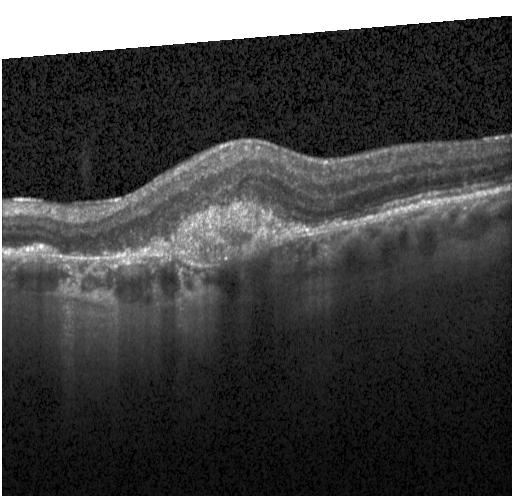 Heidelberg Spectralis · retinal OCT B-scan · SD-OCT.
Finding: a choroidal neovascular membrane.